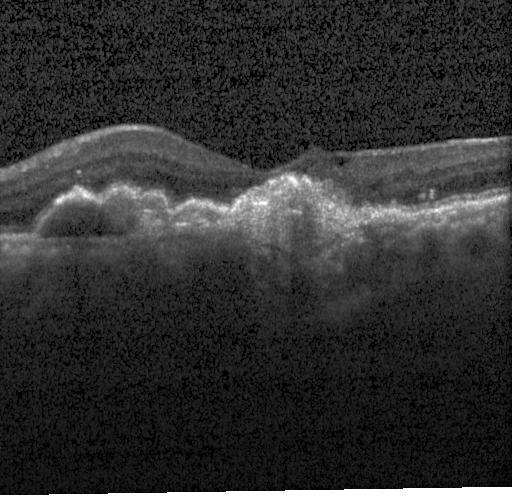

CNV.